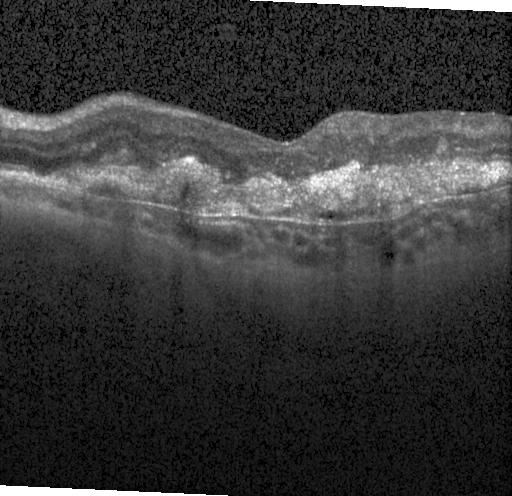

OCT finding: a choroidal neovascular membrane.